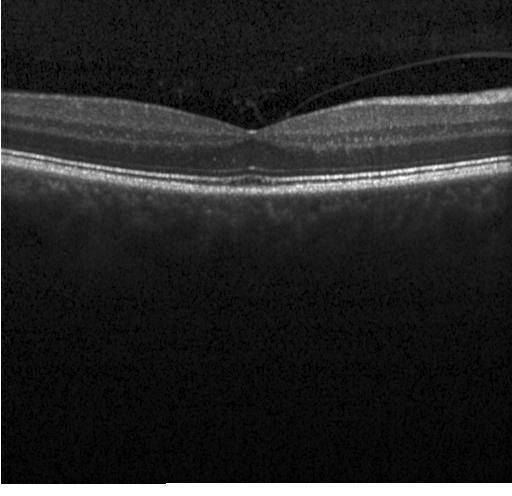
Through the macula. OCT line scan.
No choroidal neovascularization, diabetic macular edema, or drusen.